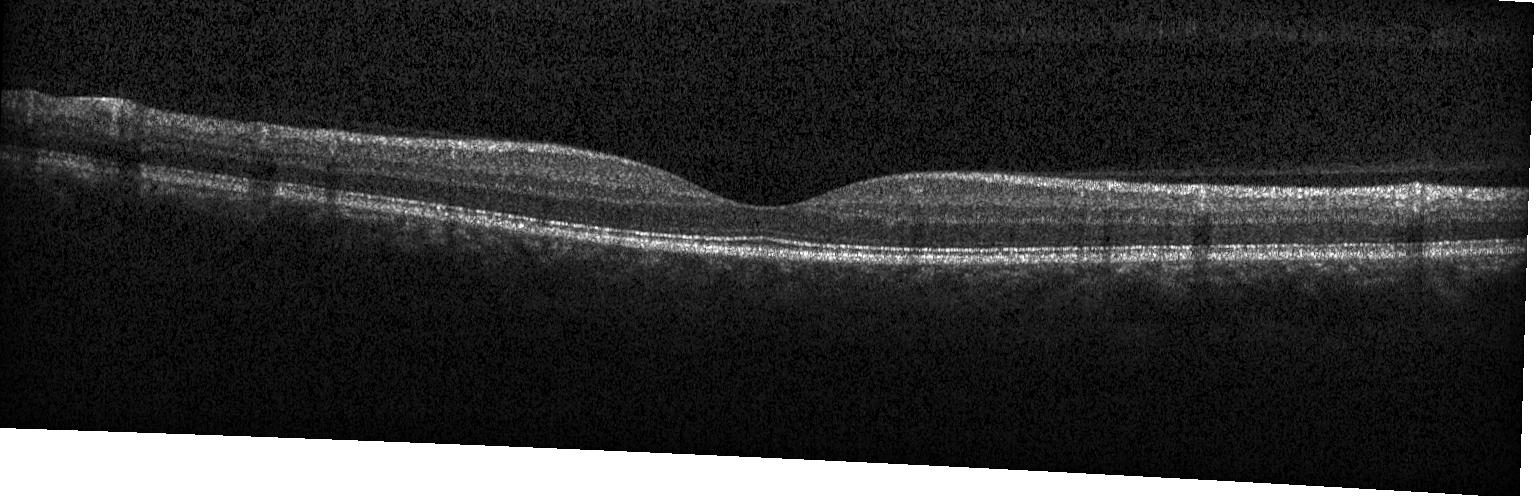

Macular scan; retinal OCT cross-section — Finding: no choroidal neovascularization, no diabetic macular edema, and no drusen.